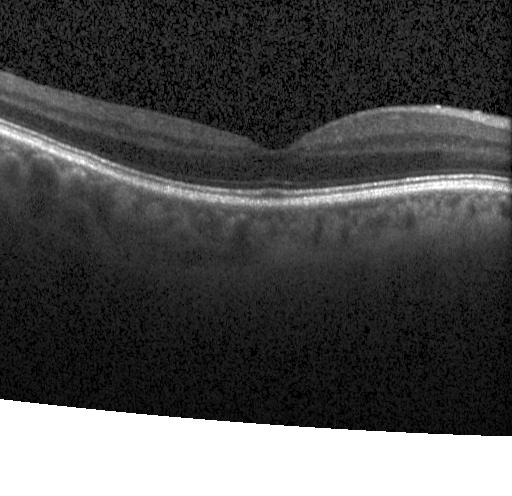

Fovea-centered; OCT B-scan.
Impression: no CNV, DME, or drusen.